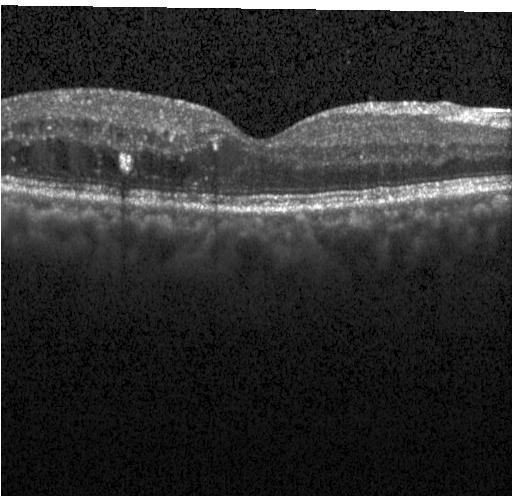 Horizontal scan through the fovea · Heidelberg Spectralis · retinal OCT B-scan.
Finding: diabetic macular edema.